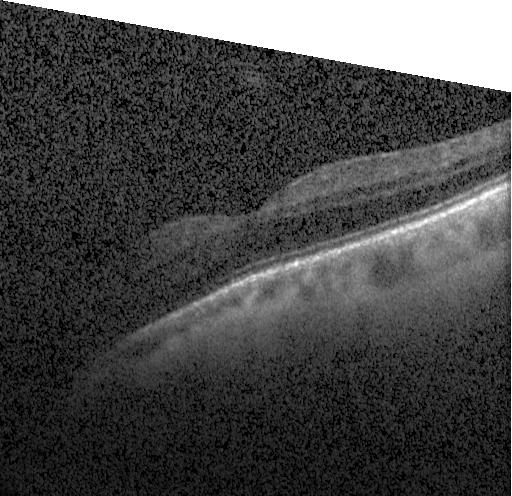 This B-scan demonstrates no choroidal neovascularization, no diabetic macular edema, and no drusen.